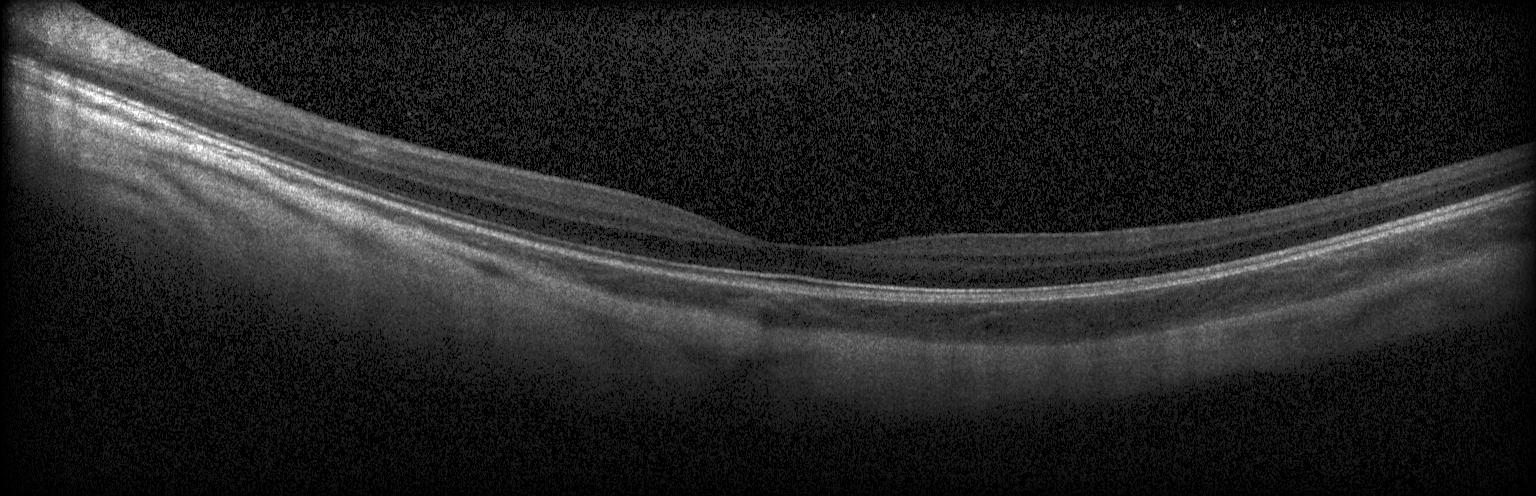

Diagnosis: no CNV, DME, or drusen.